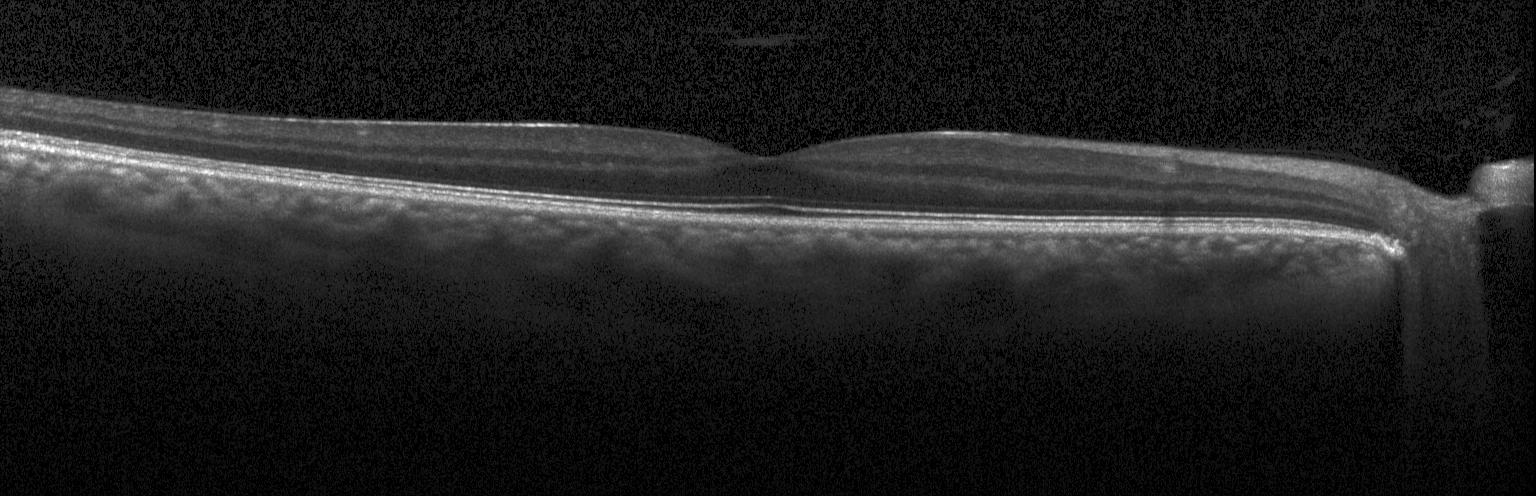 Assessment: neither choroidal neovascularization, diabetic macular edema, nor drusen.